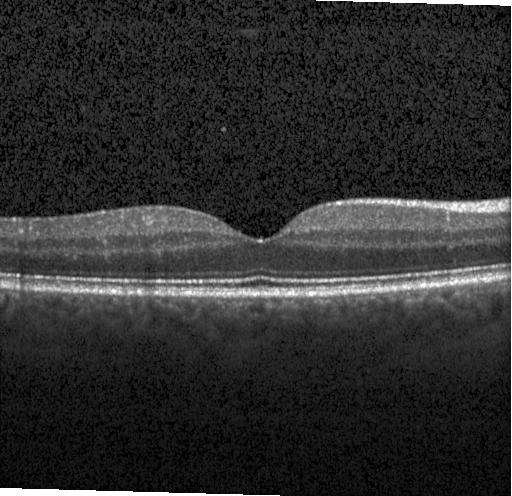

Through the macula; optical coherence tomography B-scan; spectral-domain OCT; instrument: Heidelberg Spectralis
This B-scan demonstrates no choroidal neovascularization, diabetic macular edema, or drusen.